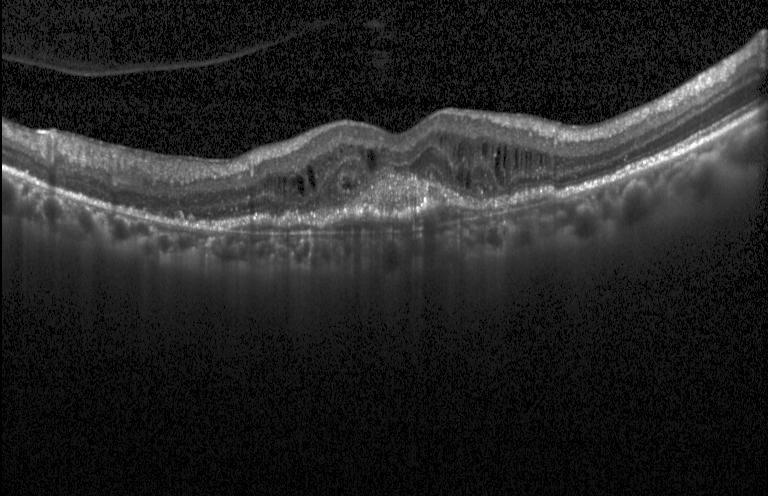 OCT line scan — The scan shows a choroidal neovascular membrane.